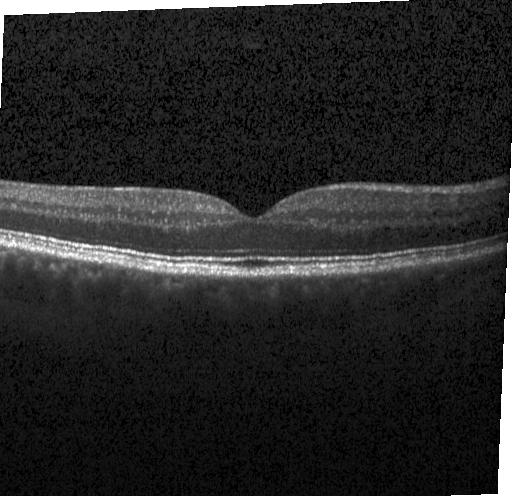

Macular scan, spectral-domain optical coherence tomography, acquired on a Heidelberg Spectralis, OCT B-scan
The scan shows no choroidal neovascularization, no diabetic macular edema, and no drusen.